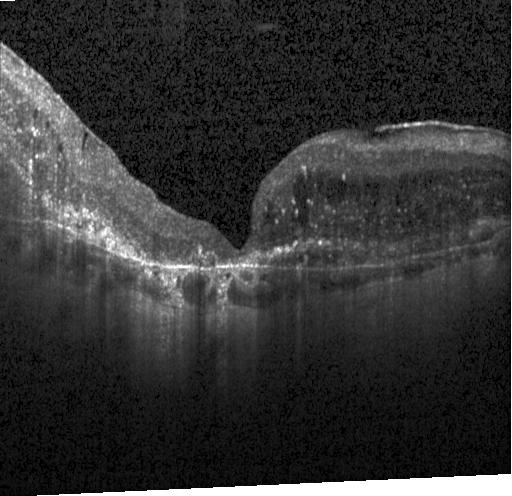 The scan shows a choroidal neovascular membrane.